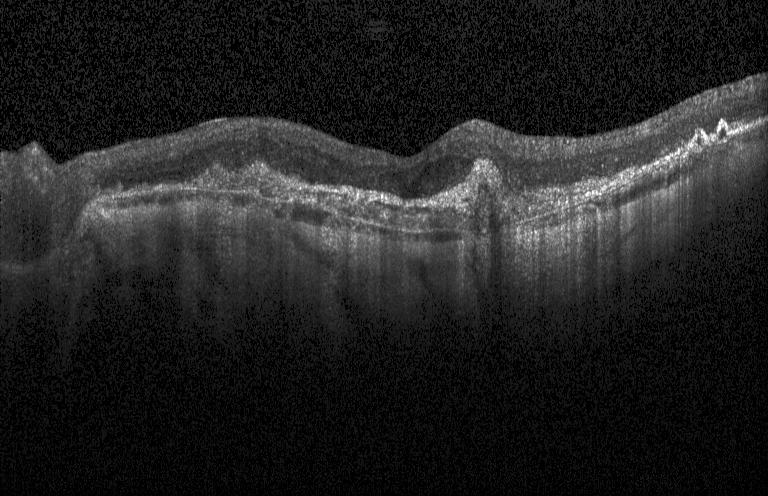

Diagnosis: CNV.